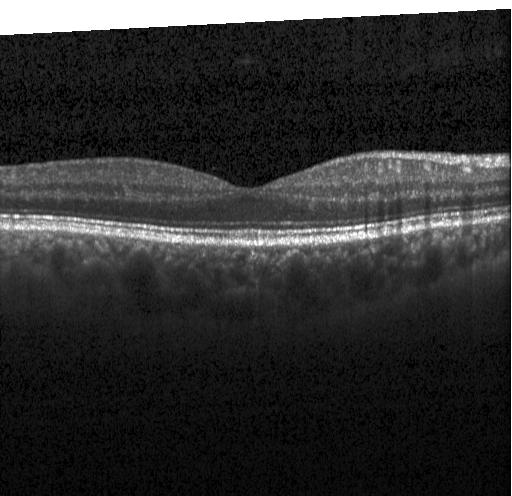

Spectral-domain OCT; macular scan; Heidelberg Spectralis OCT system; retinal OCT B-scan — Finding: no evidence of CNV, DME, or drusen.